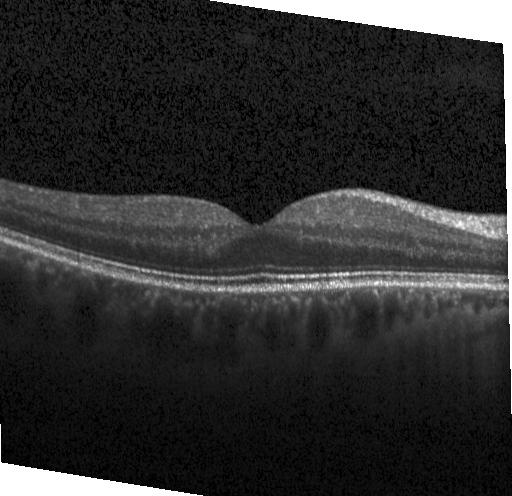
Retinal OCT cross-section showing no choroidal neovascularization, no diabetic macular edema, and no drusen.